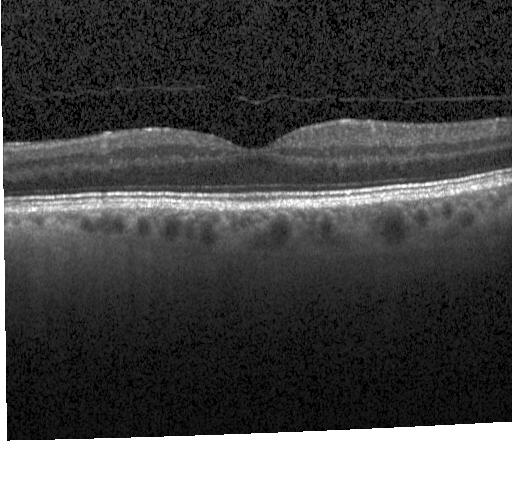
Finding: neither CNV, DME, nor drusen.